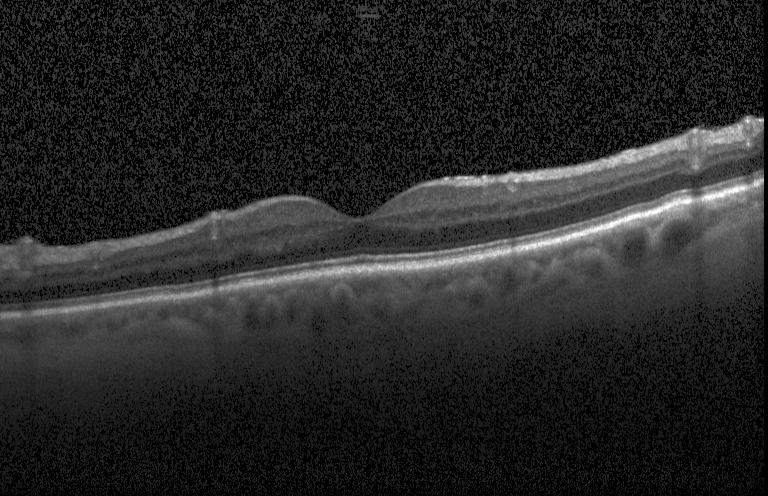
Retinal OCT B-scan. Heidelberg Spectralis
Impression: no evidence of choroidal neovascularization, diabetic macular edema, or drusen.